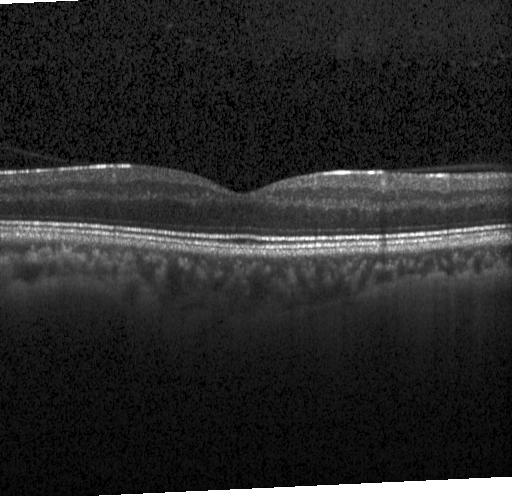

Diagnosis: neither choroidal neovascularization, diabetic macular edema, nor drusen.